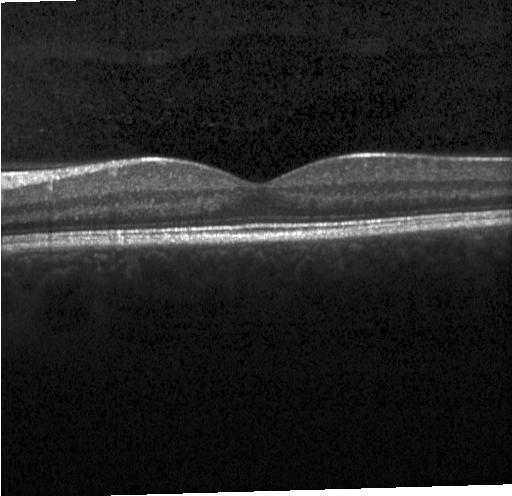 Finding: no evidence of choroidal neovascularization, diabetic macular edema, or drusen.